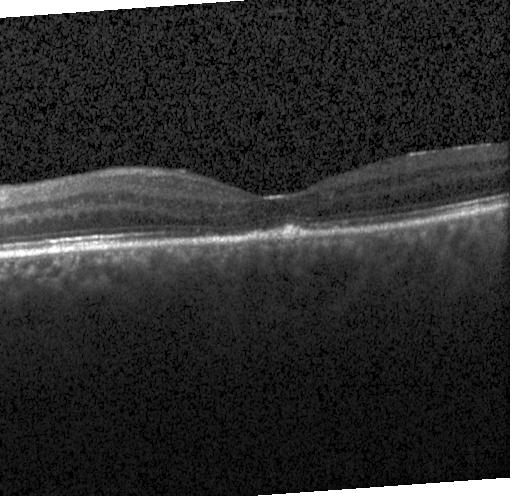

Impression: drusen.